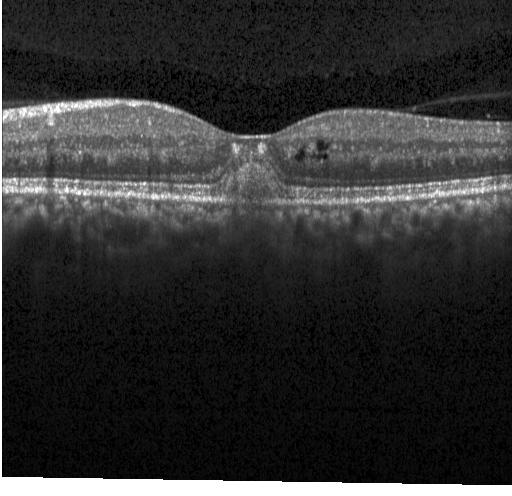 OCT line scan; centered on the fovea
A choroidal neovascular membrane.